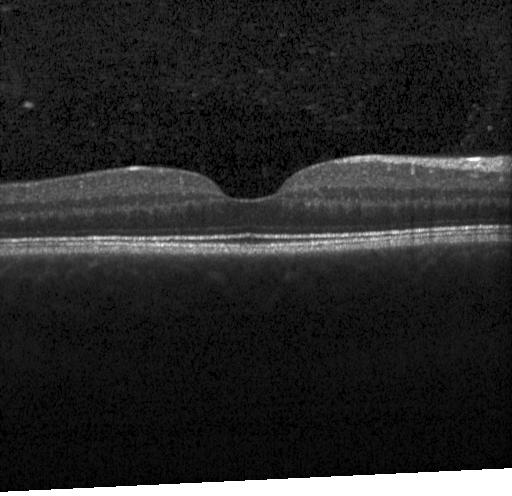
Spectral-domain optical coherence tomography · through the macula · OCT B-scan.
No CNV, no DME, and no drusen.